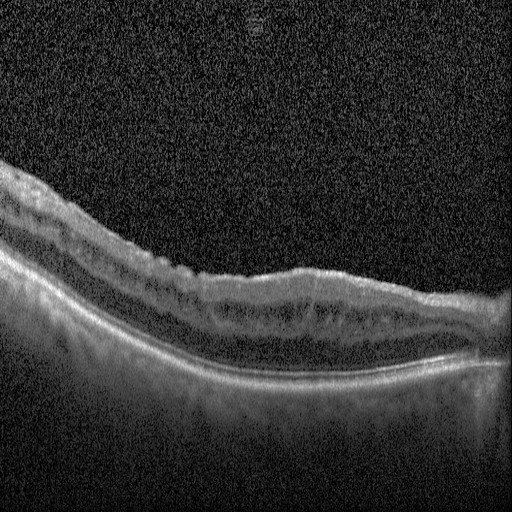

Heidelberg Spectralis · horizontal scan through the fovea · spectral-domain optical coherence tomography · optical coherence tomography scan. Dx: DME.